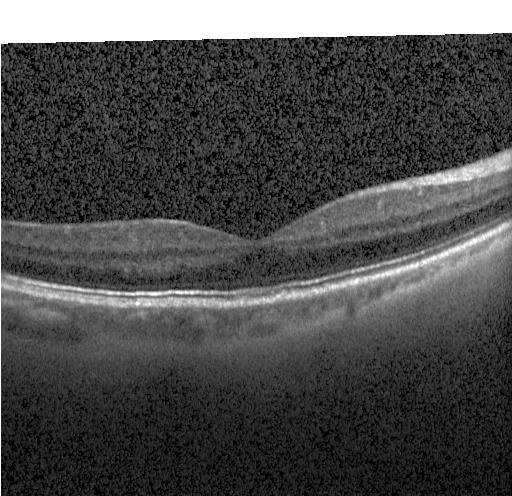 Fovea-centered, spectral-domain OCT, OCT B-scan, acquired on a Heidelberg Spectralis.
Macular OCT: no evidence of CNV, DME, or drusen.